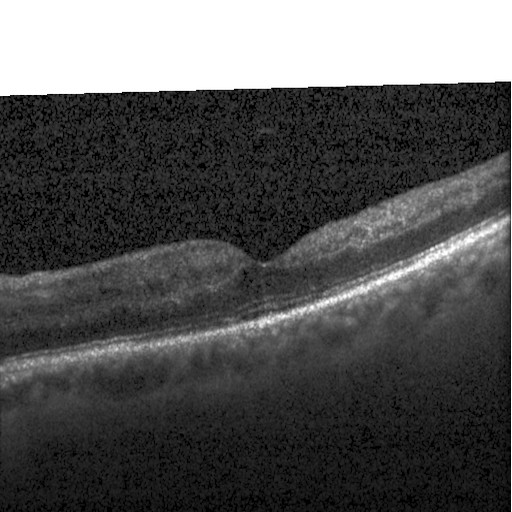 Retinal OCT cross-section — Finding: DME.